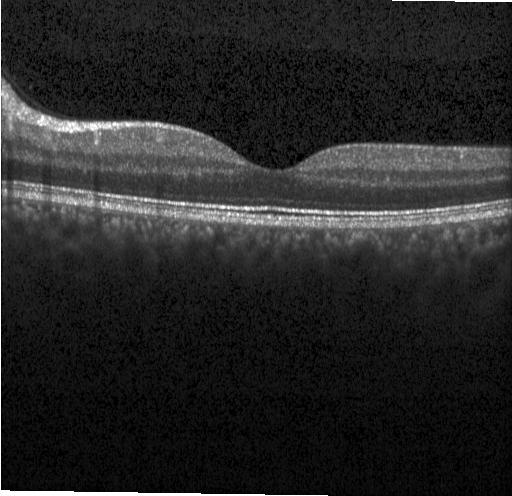 SD-OCT; Heidelberg Spectralis; through the macula; retinal OCT cross-section. OCT finding: no evidence of choroidal neovascularization, diabetic macular edema, or drusen.